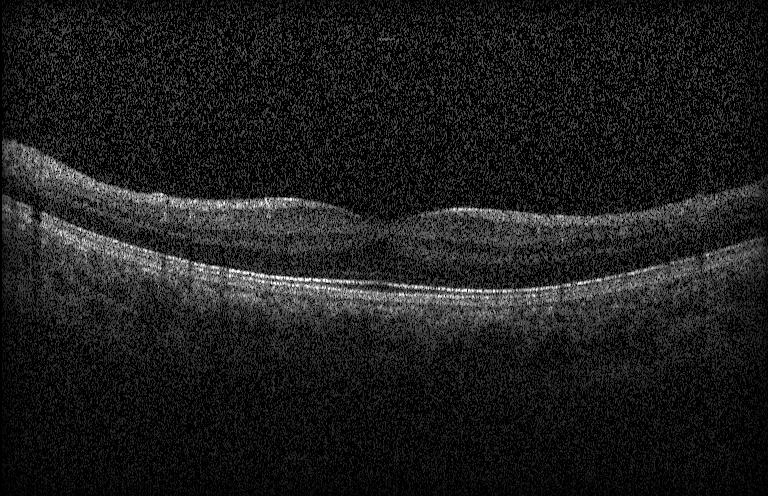 Retinal OCT B-scan — Macular OCT: no choroidal neovascularization, diabetic macular edema, or drusen.